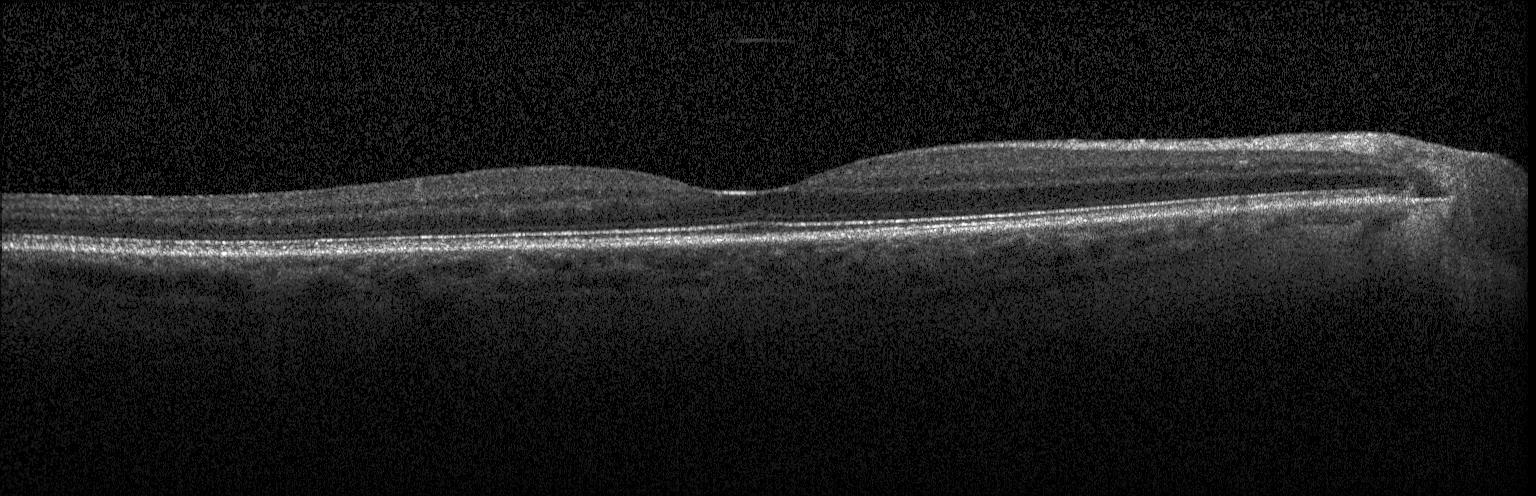 Diagnosis: no evidence of choroidal neovascularization, diabetic macular edema, or drusen.